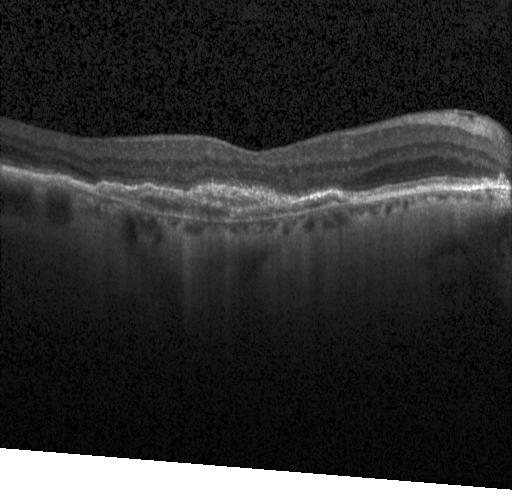 The scan shows CNV.